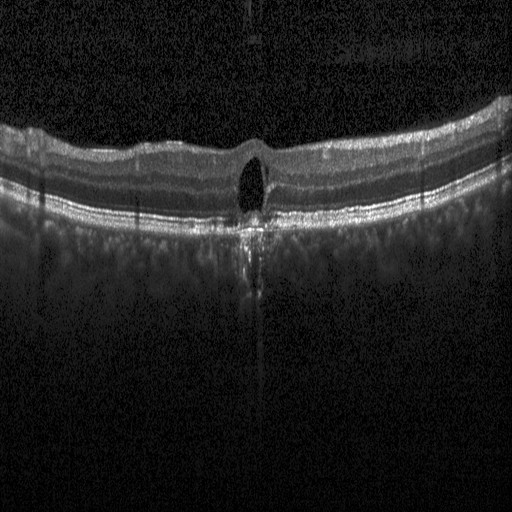
Horizontal scan through the fovea. Optical coherence tomography B-scan — Impression: diabetic macular edema (DME).